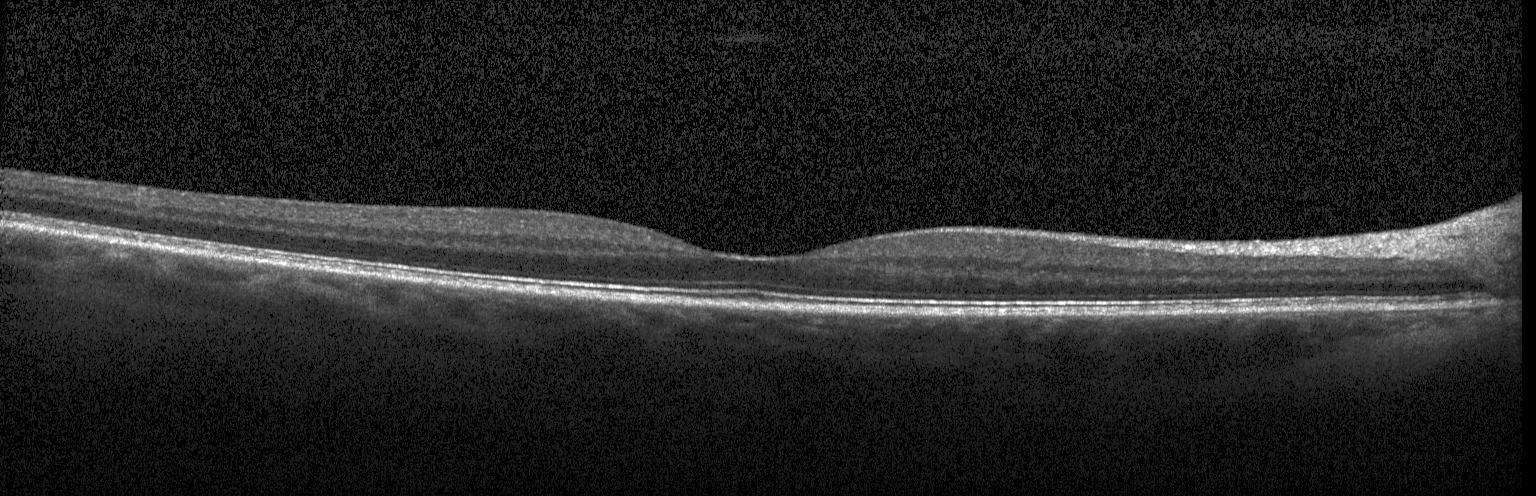 Horizontal scan through the fovea. Spectral-domain OCT. OCT B-scan.
Diagnosis: neither choroidal neovascularization, diabetic macular edema, nor drusen.